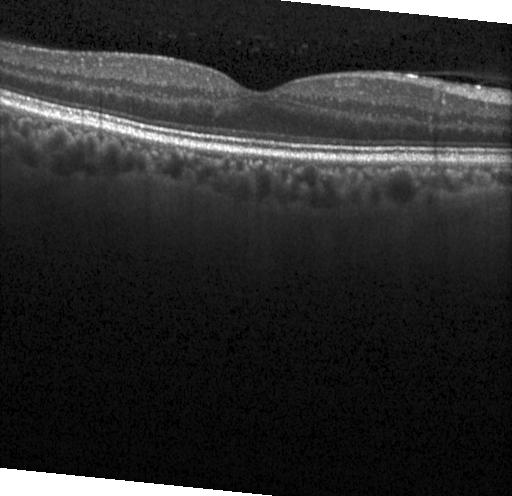
Dx: no CNV, DME, or drusen.